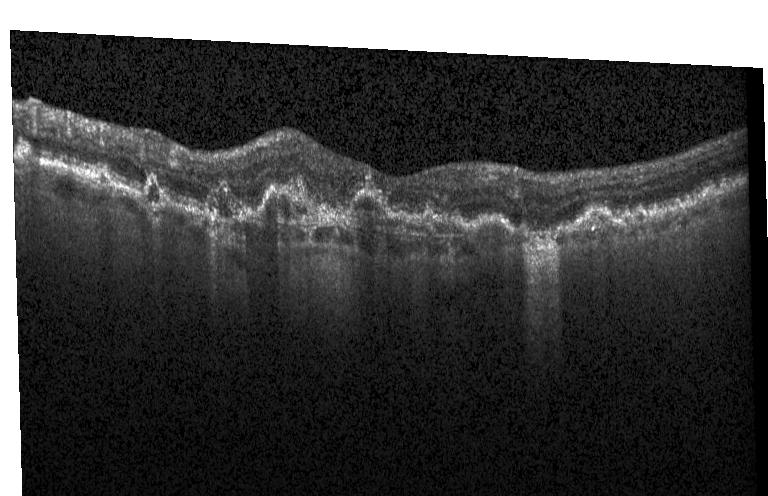 Macular OCT: choroidal neovascularization (CNV).